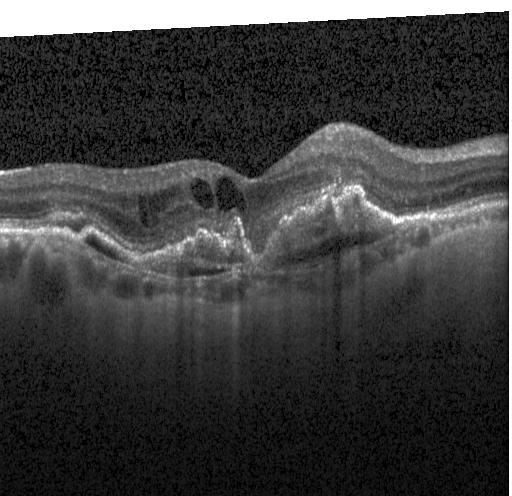

Spectral-domain optical coherence tomography, OCT line scan.
The scan shows a choroidal neovascular membrane.